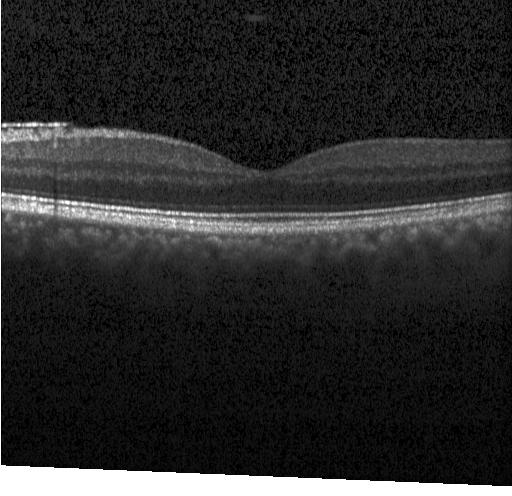
Instrument: Heidelberg Spectralis; retinal OCT cross-section.
The scan shows no choroidal neovascularization, diabetic macular edema, or drusen.